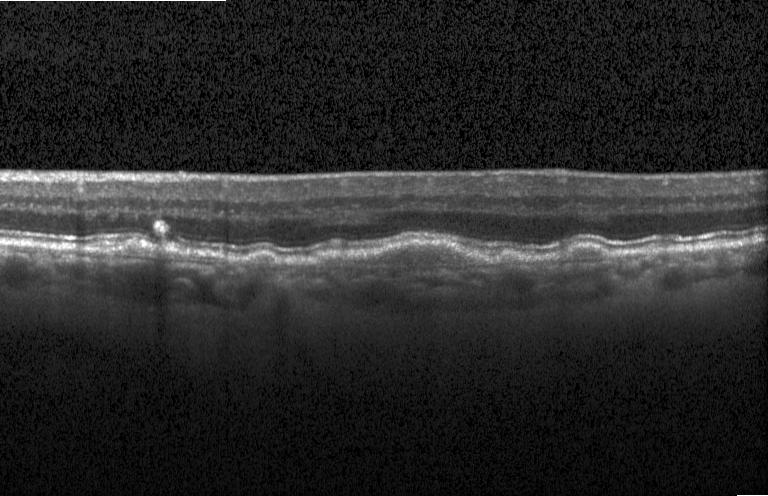 OCT B-scan. Finding: multiple drusen.